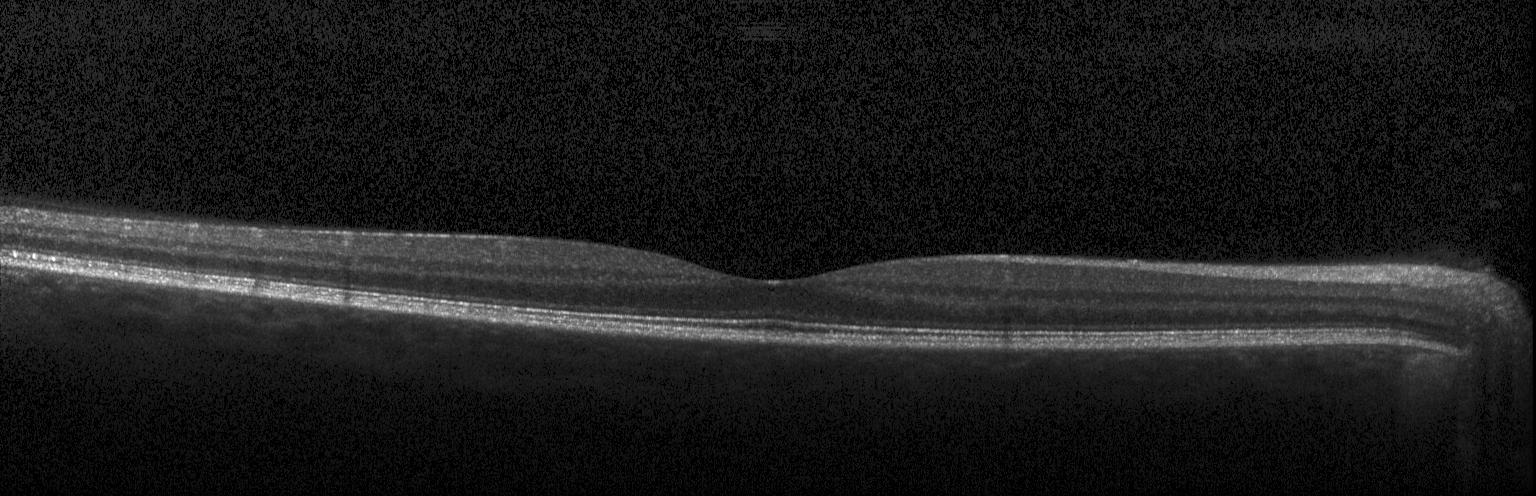 Acquired on a Heidelberg Spectralis, SD-OCT, optical coherence tomography scan. Finding: no CNV, DME, or drusen.